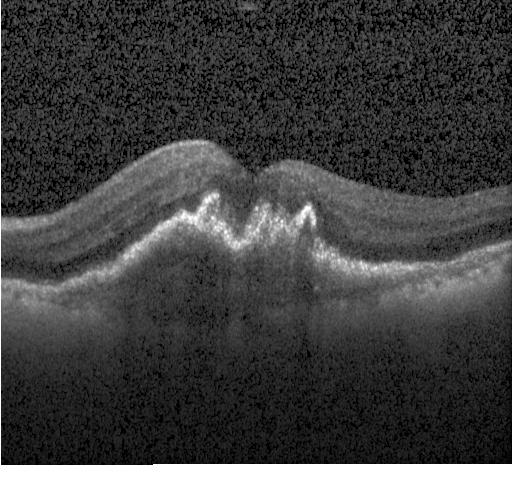

Optical coherence tomography B-scan · spectral-domain OCT · instrument: Heidelberg Spectralis · through the macula.
Macular OCT: a choroidal neovascular membrane.